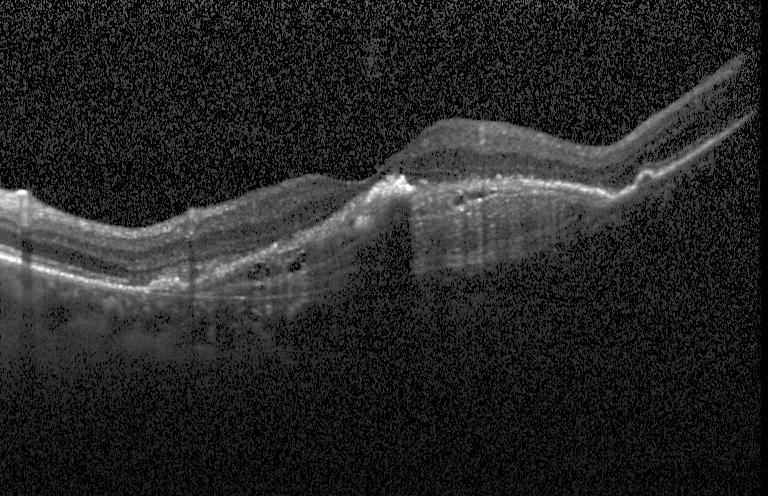

Choroidal neovascularization (CNV).